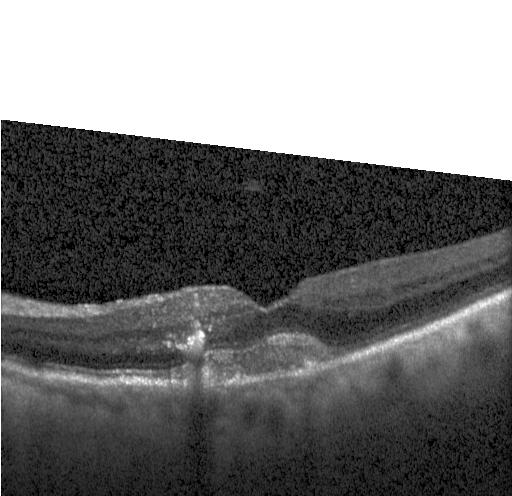
Horizontal scan through the fovea · optical coherence tomography B-scan · Heidelberg Spectralis
Dx: choroidal neovascularization.